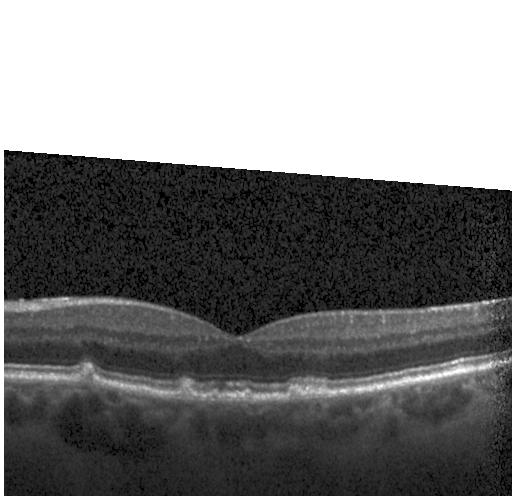
OCT B-scan showing multiple drusen.